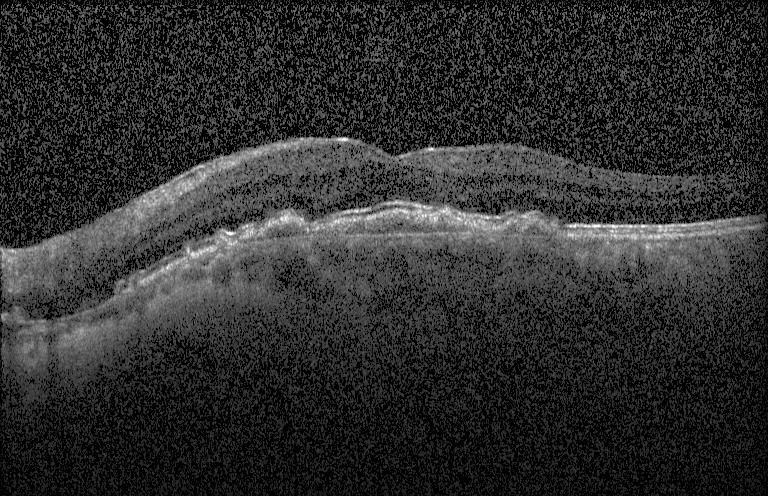
Retinal OCT B-scan. This B-scan demonstrates a choroidal neovascular membrane.